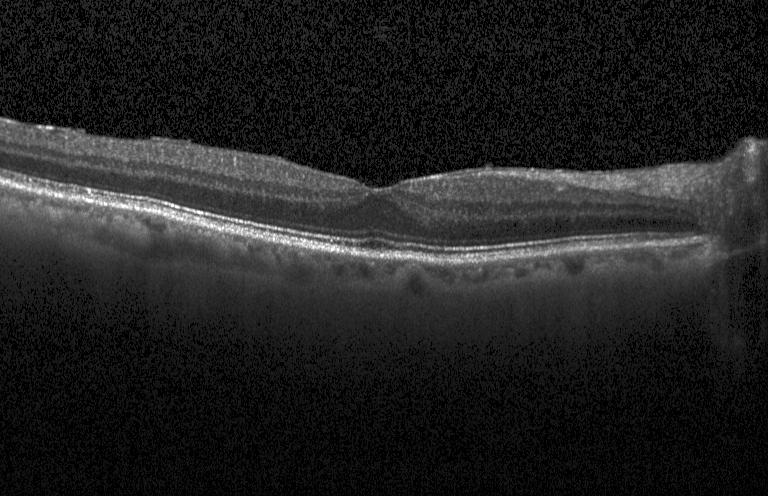

OCT finding: neither choroidal neovascularization, diabetic macular edema, nor drusen.